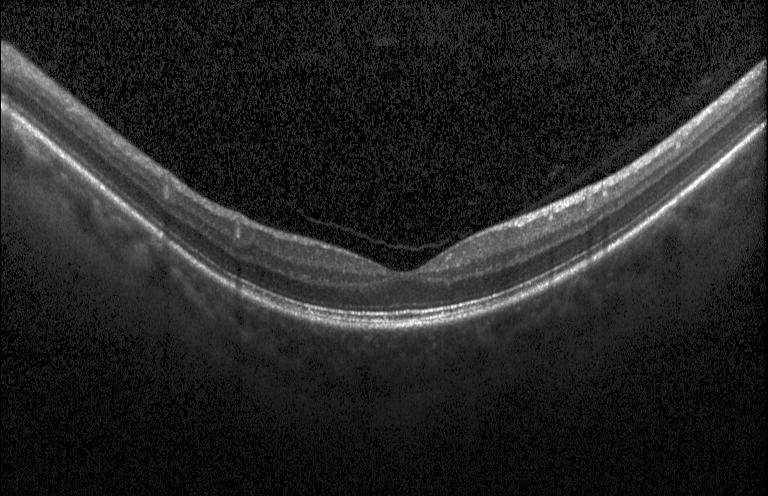

Finding: no evidence of CNV, DME, or drusen.